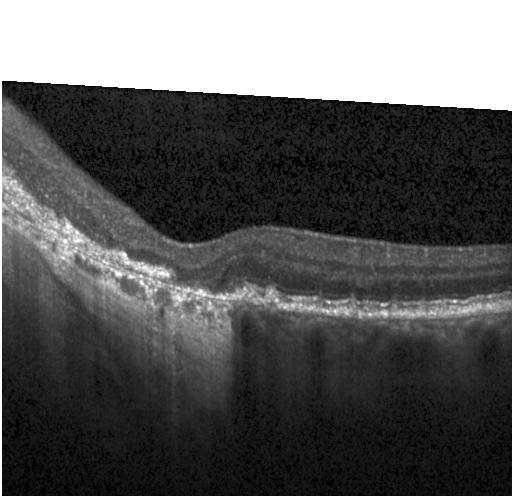 Acquired on a Heidelberg Spectralis; optical coherence tomography scan; centered on the fovea. Finding: choroidal neovascularization (CNV).